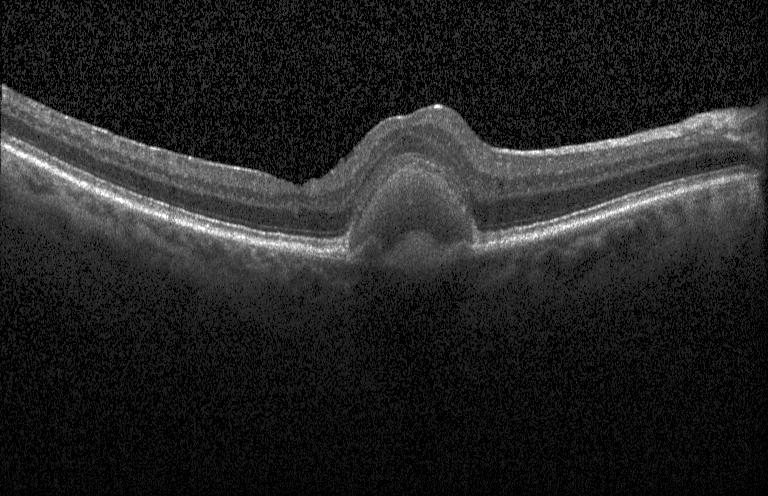

Diagnosis: a choroidal neovascular membrane.